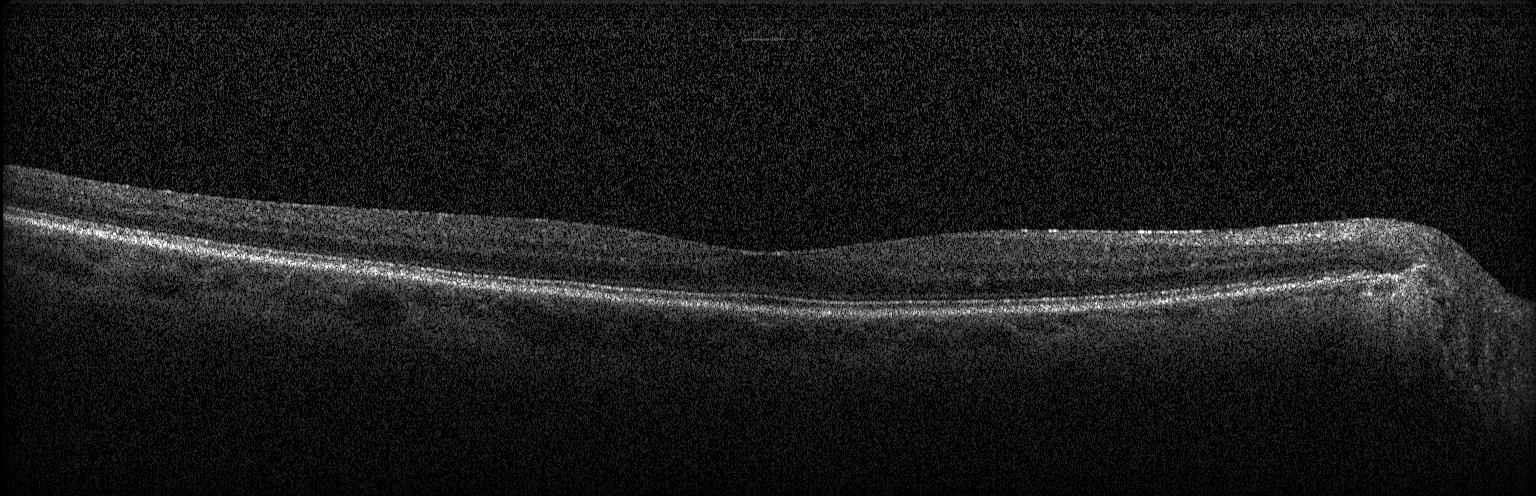

Instrument: Heidelberg Spectralis · retinal OCT B-scan — Diagnosis: no choroidal neovascularization, no diabetic macular edema, and no drusen.